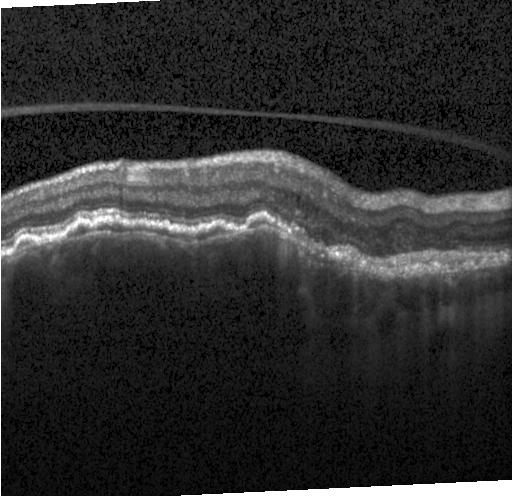
Retinal OCT B-scan. Acquired on a Heidelberg Spectralis. Spectral-domain OCT. Centered on the fovea. Finding: a choroidal neovascular membrane.